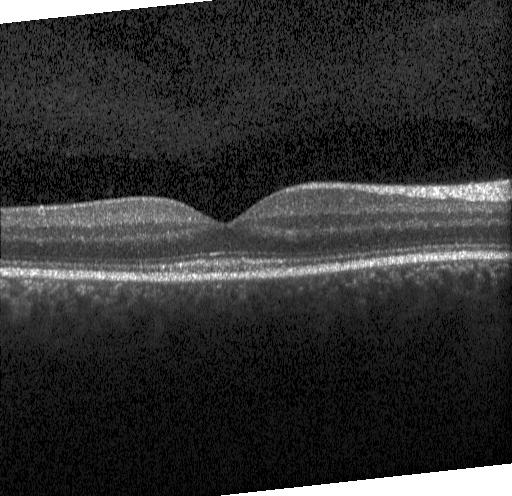

Macular OCT: no evidence of CNV, DME, or drusen.